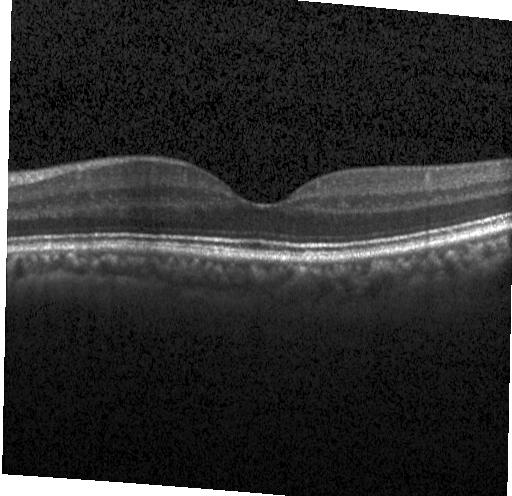
Macular OCT: no evidence of CNV, DME, or drusen.